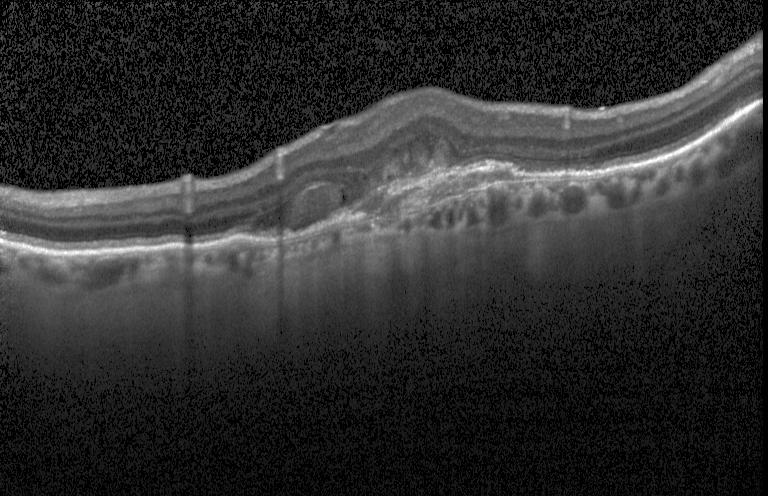

Finding: choroidal neovascularization.